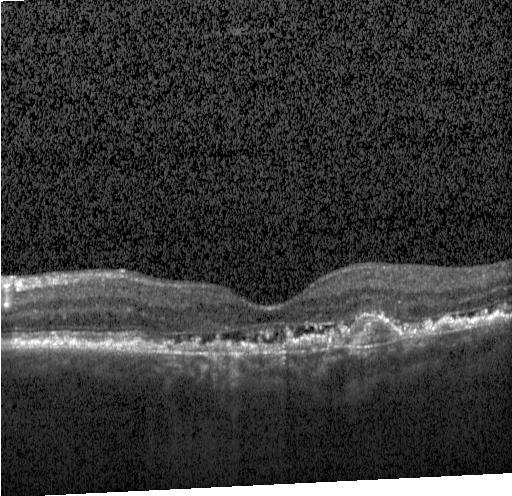
Impression: choroidal neovascularization (CNV).